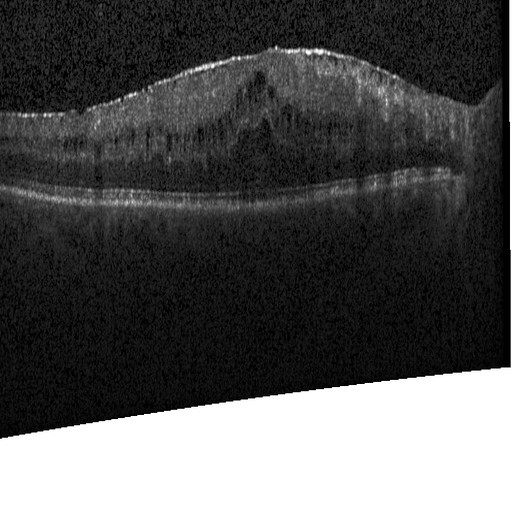 Finding: diabetic macular edema (DME).